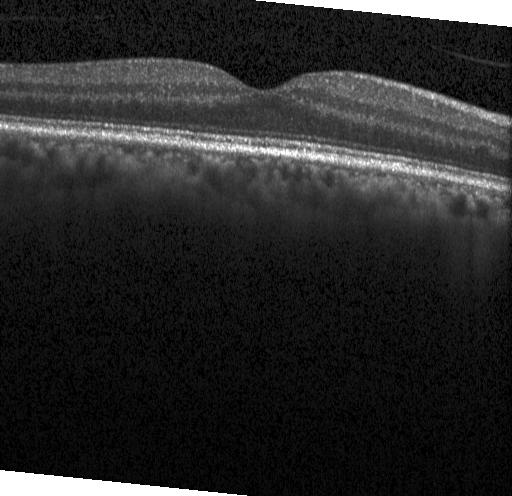

OCT B-scan; through the macula; spectral-domain optical coherence tomography
Finding: no CNV, no DME, and no drusen.